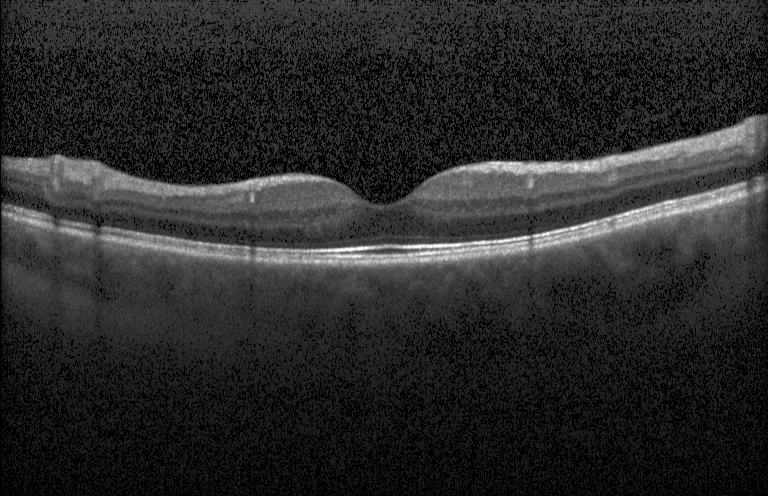

Spectral-domain OCT. Macular scan. Acquired on a Heidelberg Spectralis. Retinal OCT B-scan — Finding: neither CNV, DME, nor drusen.